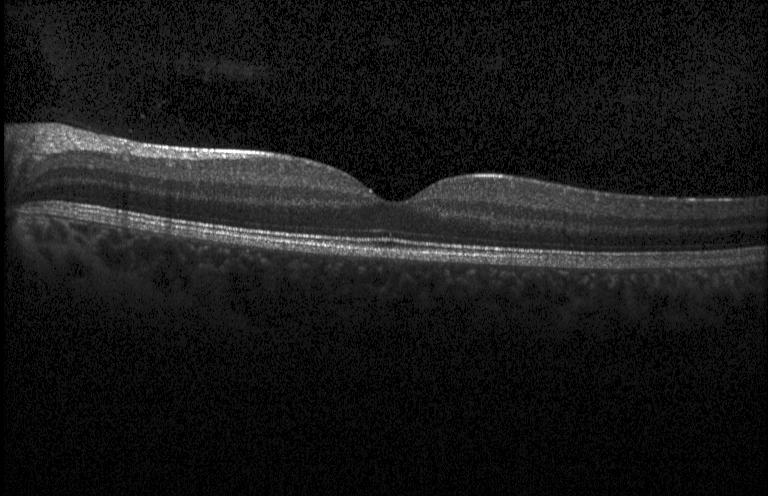

OCT finding: no evidence of choroidal neovascularization, diabetic macular edema, or drusen.